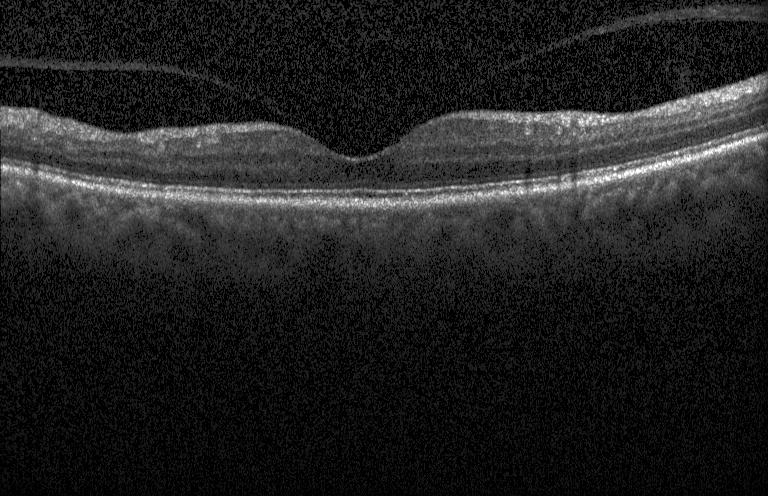
OCT line scan, fovea-centered.
Macular OCT: no choroidal neovascularization, diabetic macular edema, or drusen.